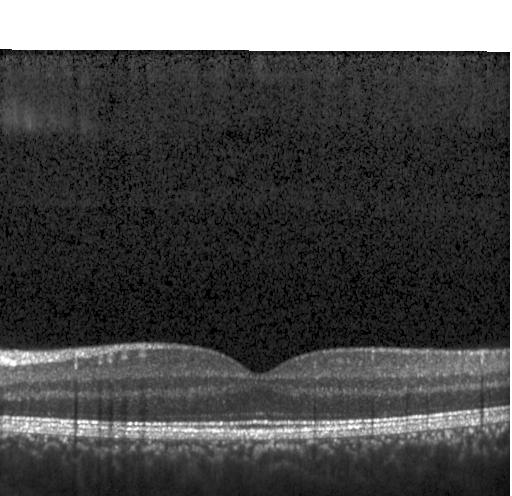

Optical coherence tomography scan, Heidelberg Spectralis — Impression: no CNV, DME, or drusen.